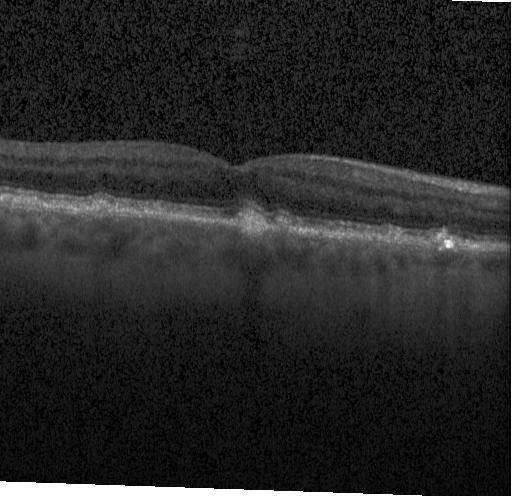
Optical coherence tomography scan, spectral-domain optical coherence tomography, macular scan, Heidelberg Spectralis.
Impression: drusen.